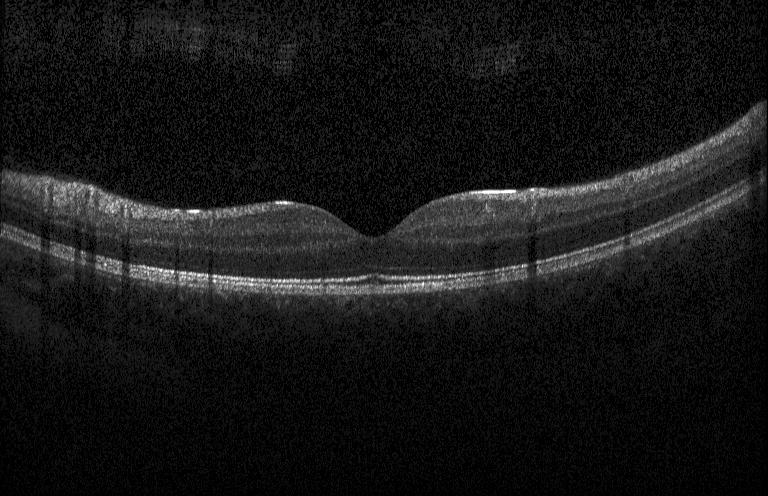
OCT finding: neither CNV, DME, nor drusen.